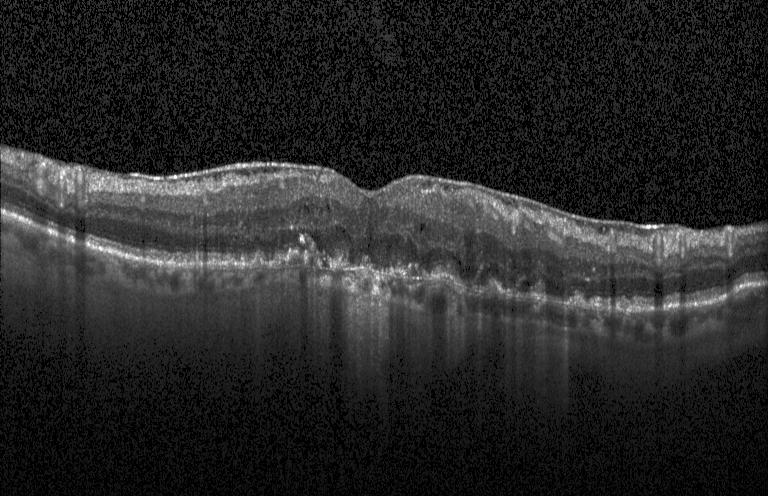
A choroidal neovascular membrane.